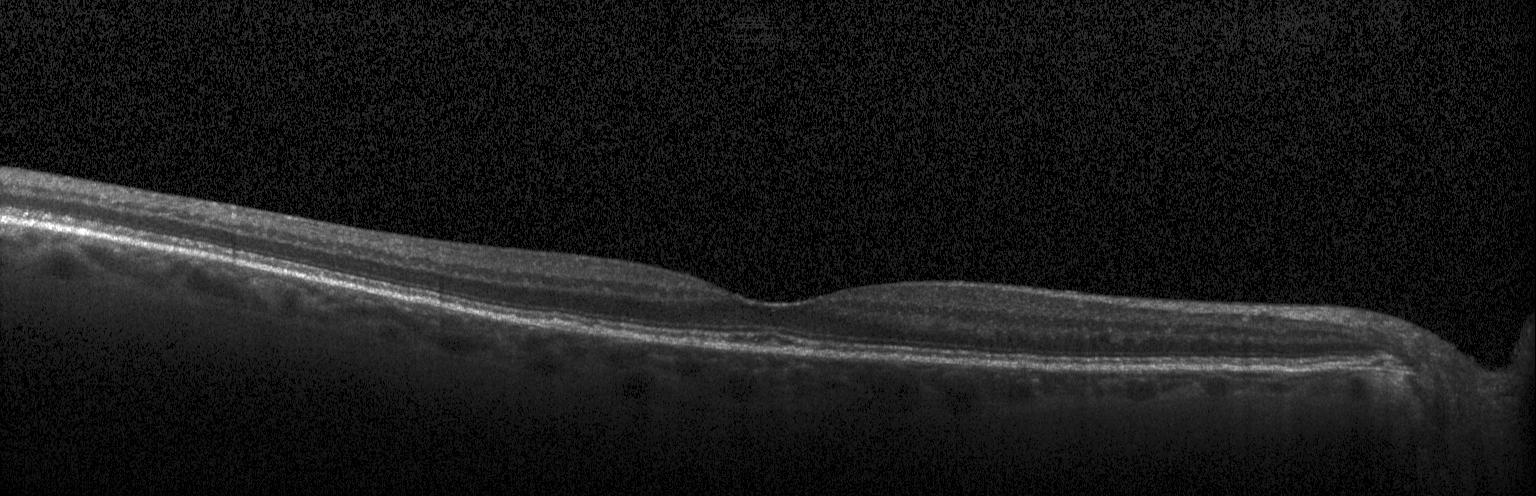

Instrument: Heidelberg Spectralis. Retinal OCT cross-section — Finding: neither CNV, DME, nor drusen.